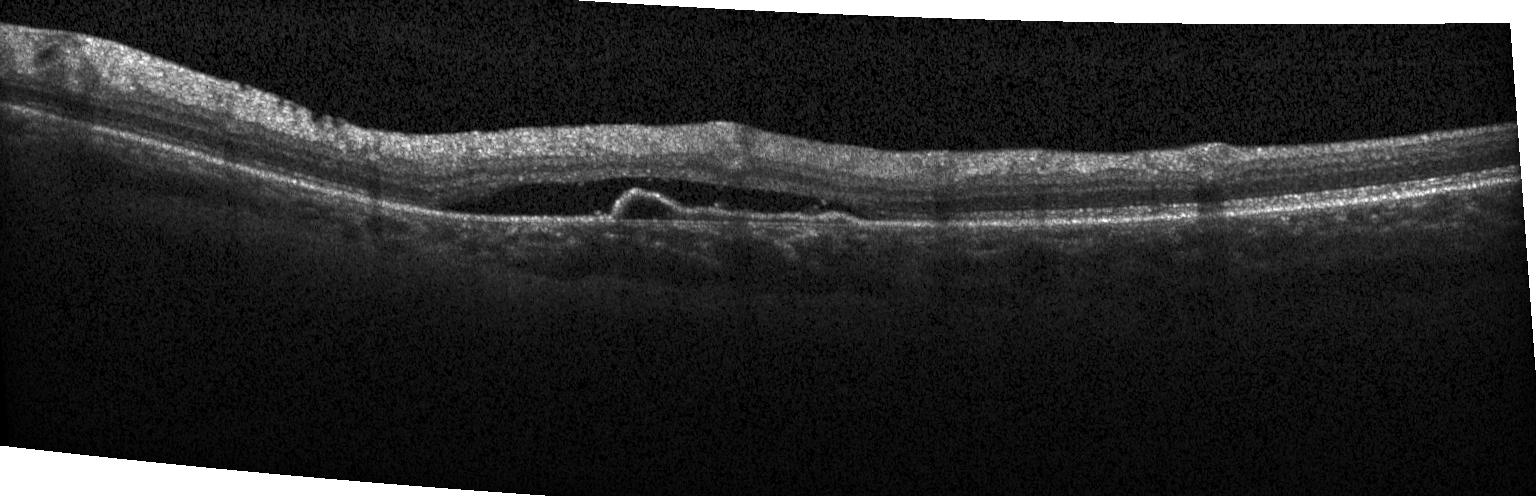 Finding: CNV.